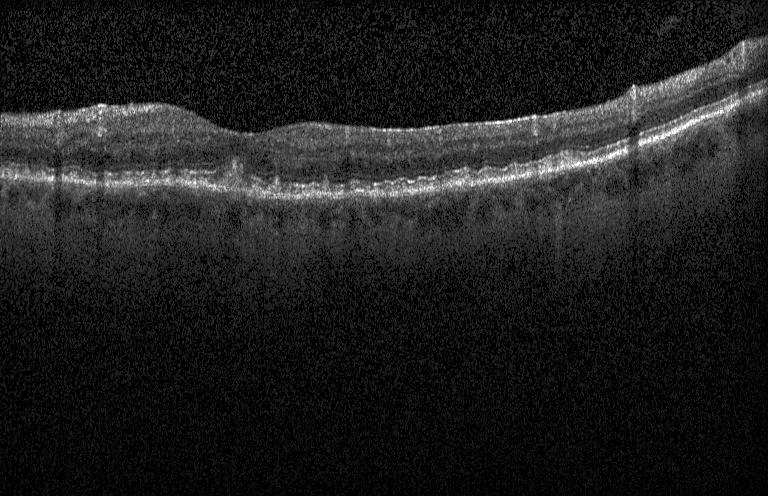

Dx: drusen.